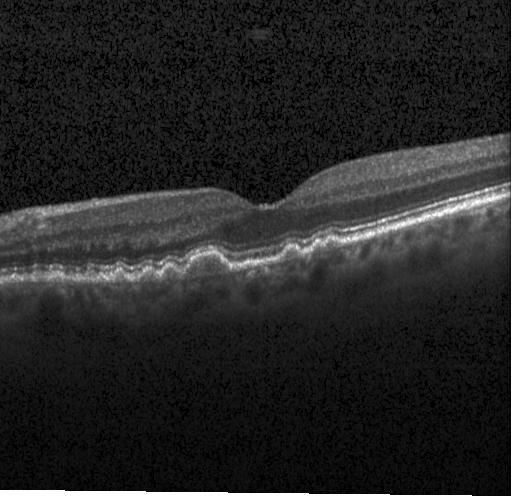 Macular scan · optical coherence tomography scan.
Diagnosis: drusen.